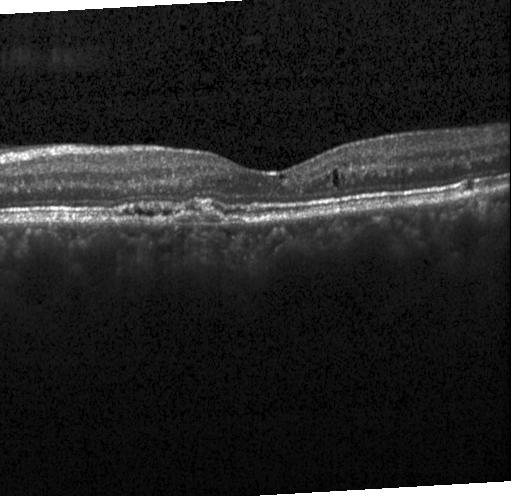 OCT line scan.
Finding: a choroidal neovascular membrane.